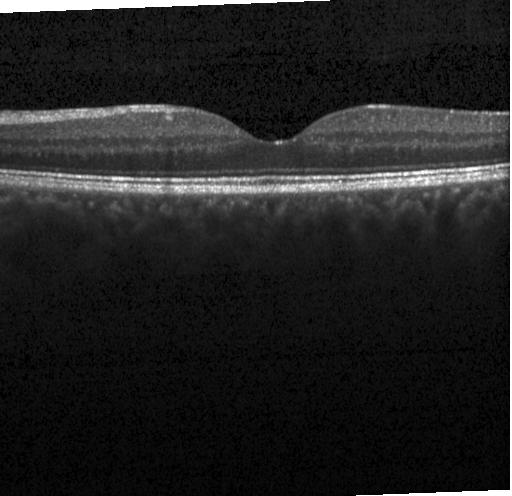
Macular OCT: neither choroidal neovascularization, diabetic macular edema, nor drusen.